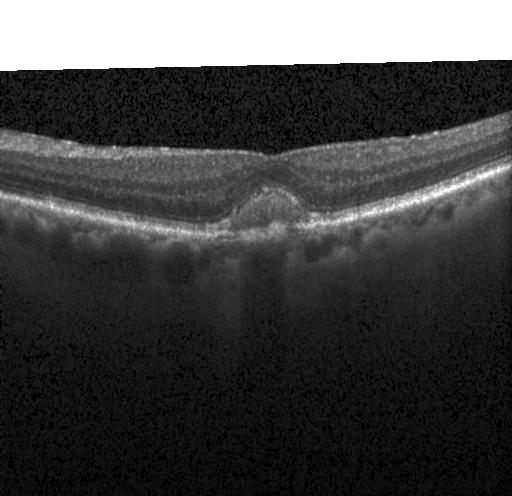

Optical coherence tomography scan · SD-OCT · instrument: Heidelberg Spectralis. Impression: a choroidal neovascular membrane.